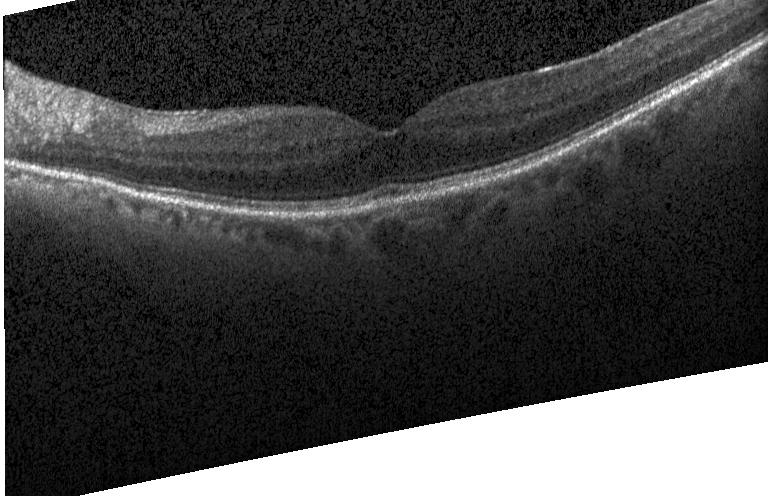
Dx: no choroidal neovascularization, diabetic macular edema, or drusen.